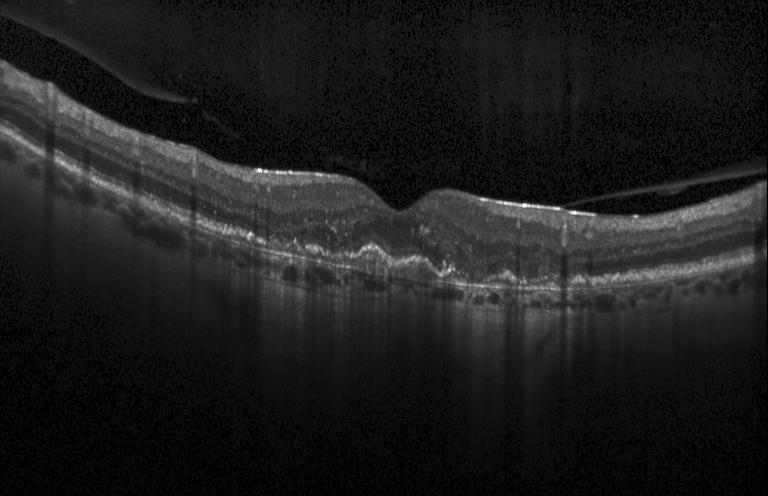
OCT B-scan, SD-OCT, Heidelberg Spectralis, centered on the fovea.
OCT finding: choroidal neovascularization.